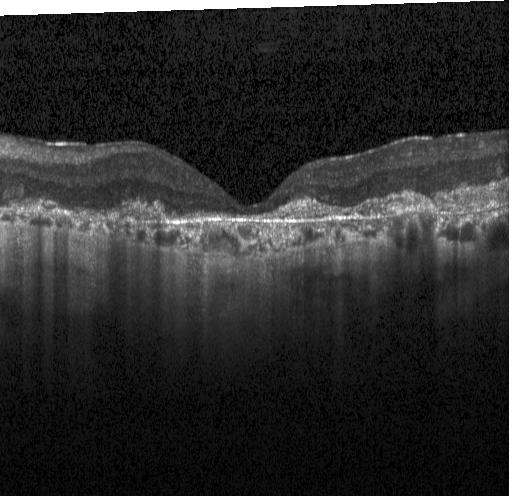

SD-OCT · horizontal scan through the fovea · retinal OCT B-scan
OCT finding: a choroidal neovascular membrane.